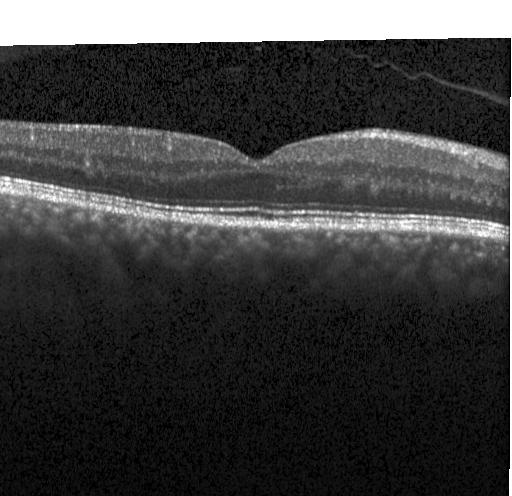 OCT finding: no evidence of choroidal neovascularization, diabetic macular edema, or drusen.